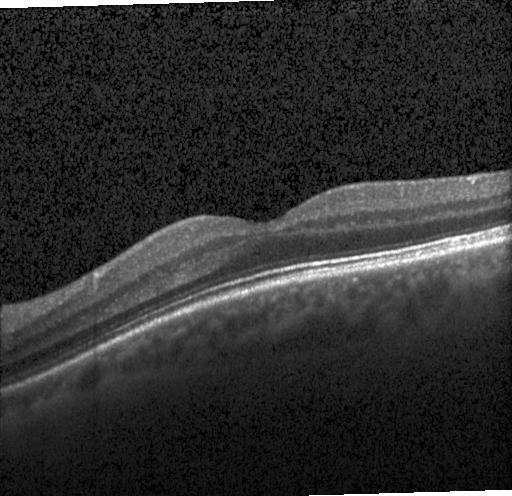
Spectral-domain optical coherence tomography · horizontal scan through the fovea · Heidelberg Spectralis · retinal OCT cross-section
Diagnosis: neither choroidal neovascularization, diabetic macular edema, nor drusen.